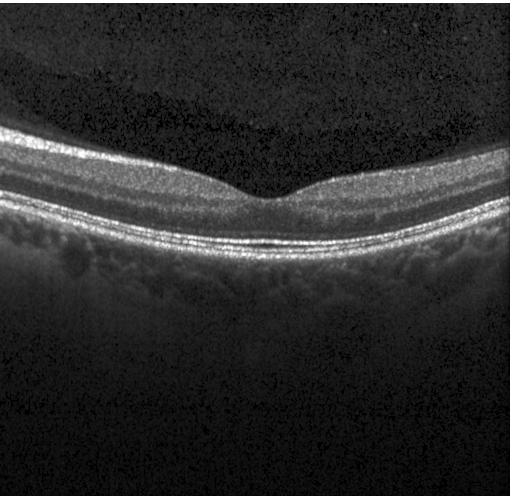 Retinal OCT cross-section showing no CNV, no DME, and no drusen.